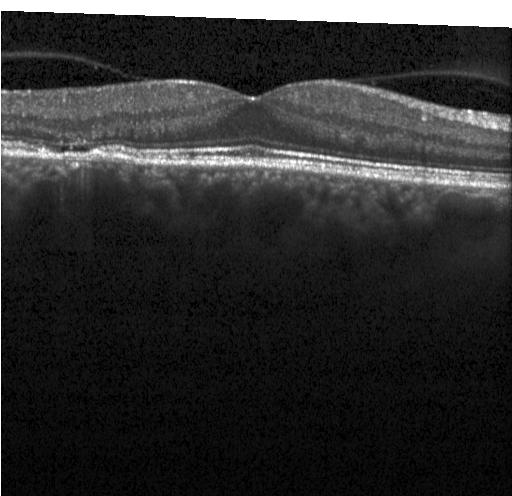
Optical coherence tomography B-scan
Assessment: choroidal neovascularization (CNV).